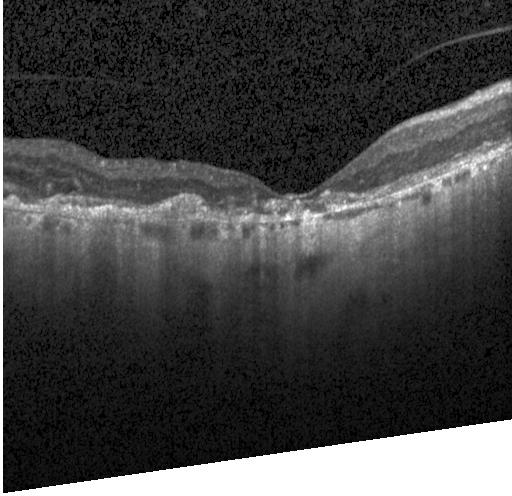 Retinal OCT cross-section, through the macula, instrument: Heidelberg Spectralis — Impression: a choroidal neovascular membrane.